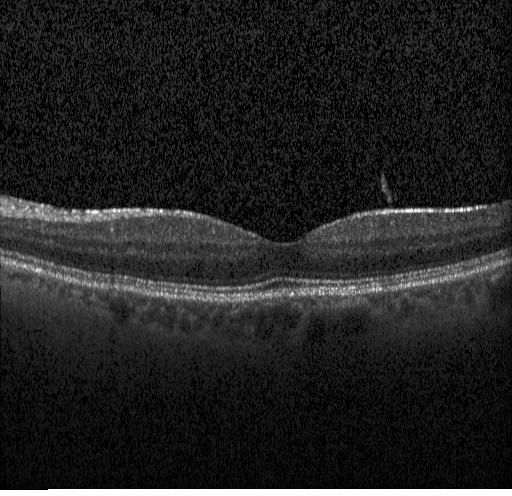

Optical coherence tomography B-scan
Finding: neither choroidal neovascularization, diabetic macular edema, nor drusen.